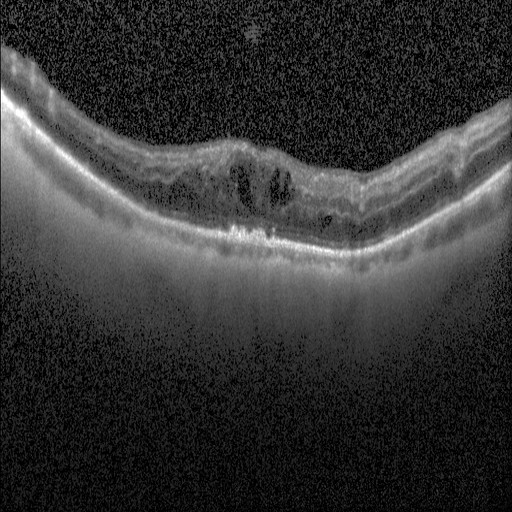

Finding: DME.